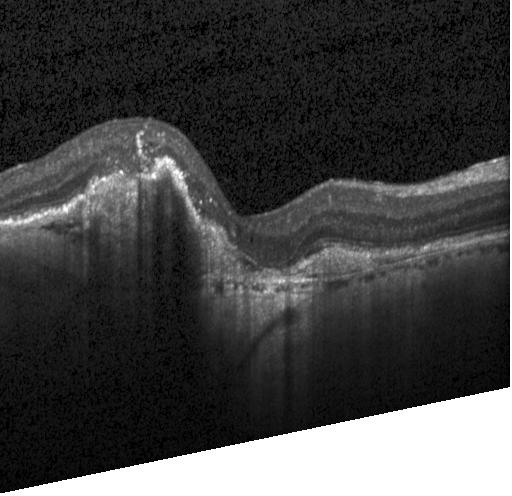
Finding: choroidal neovascularization (CNV).